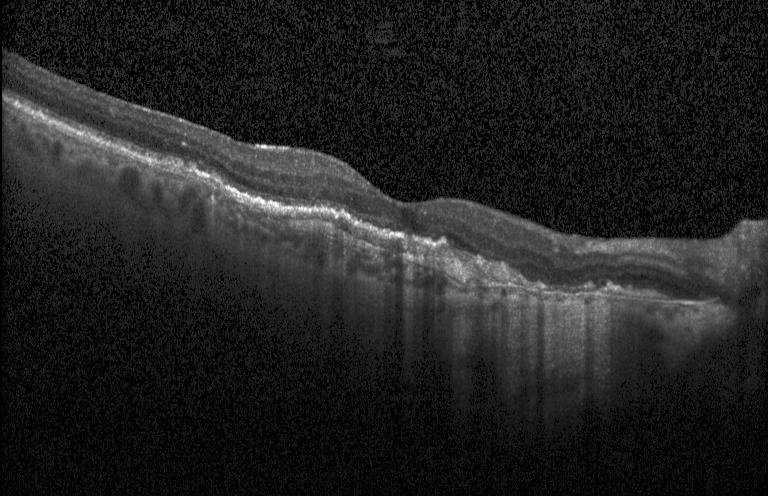 Retinal OCT cross-section; Heidelberg Spectralis; spectral-domain OCT. Finding: choroidal neovascularization.